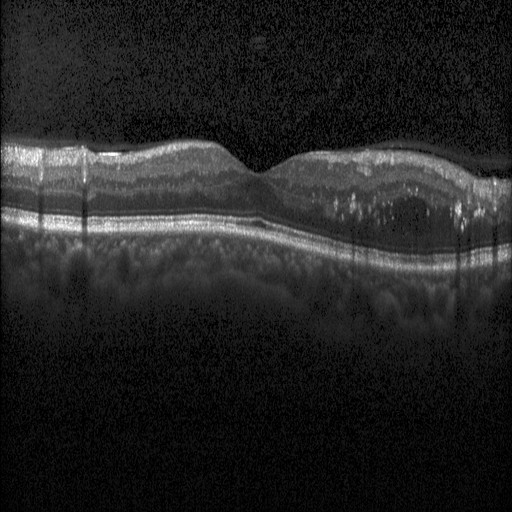
Optical coherence tomography B-scan; macular scan. Finding: diabetic macular edema (DME).